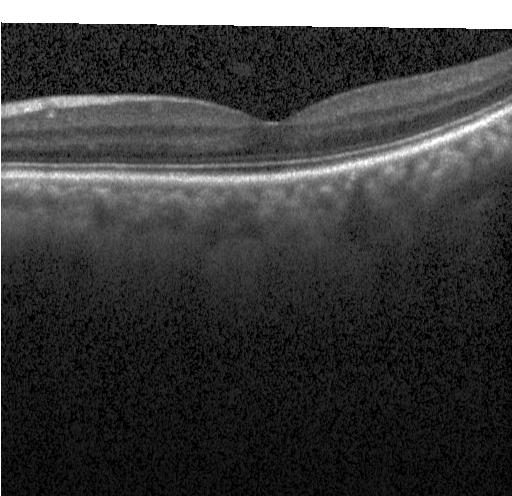
Optical coherence tomography scan; macular scan; Heidelberg Spectralis.
Neither choroidal neovascularization, diabetic macular edema, nor drusen.